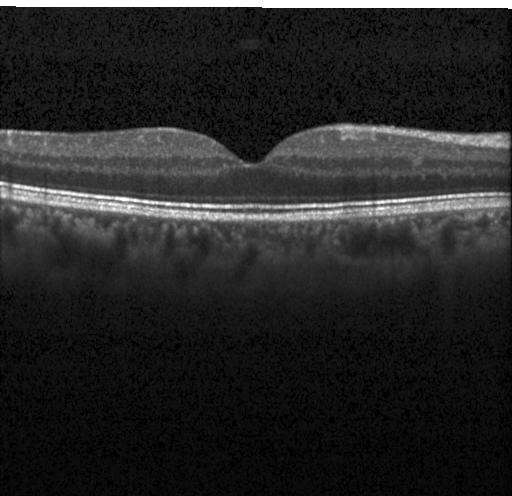

Heidelberg Spectralis OCT system. OCT line scan. Spectral-domain OCT. Assessment: no choroidal neovascularization, no diabetic macular edema, and no drusen.